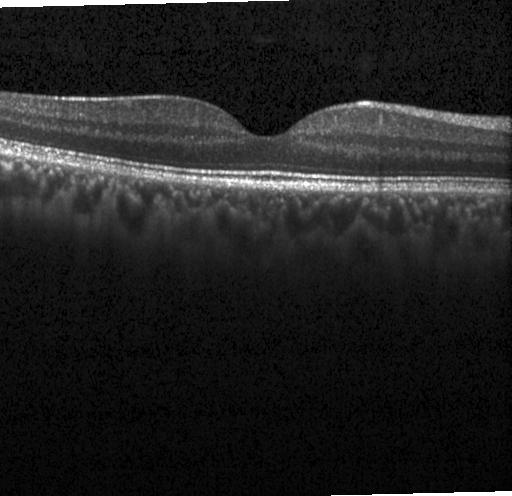

Instrument: Heidelberg Spectralis · OCT B-scan.
The scan shows no choroidal neovascularization, no diabetic macular edema, and no drusen.